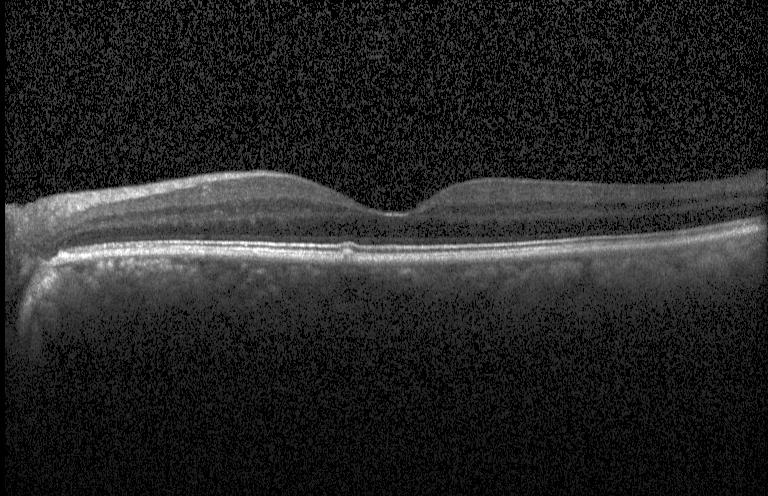 OCT B-scan showing neither choroidal neovascularization, diabetic macular edema, nor drusen.